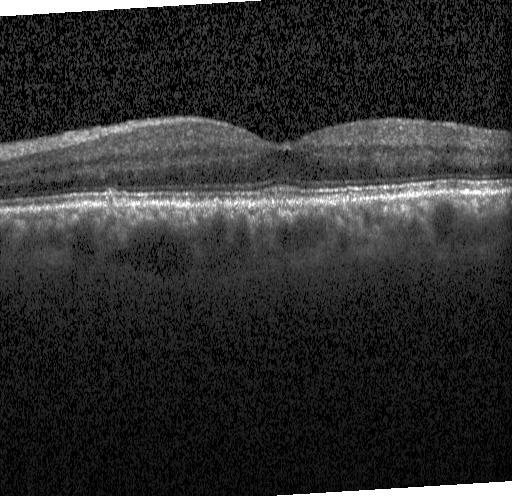 OCT B-scan. Spectral-domain optical coherence tomography.
Diagnosis: sub-RPE drusenoid deposits.